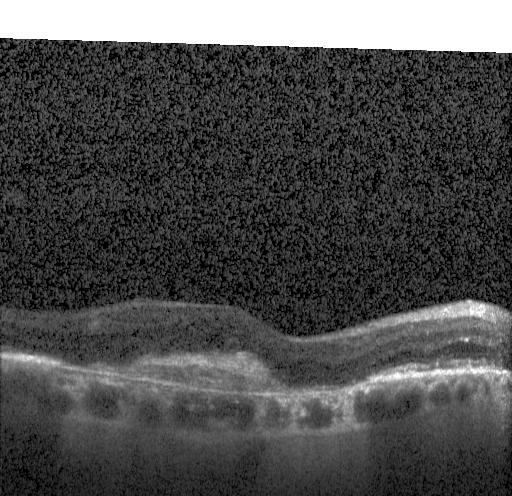
Retinal OCT B-scan
Assessment: choroidal neovascularization (CNV).